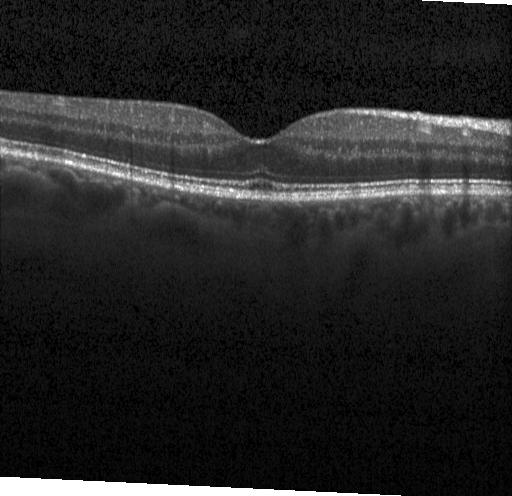

Heidelberg Spectralis OCT system · spectral-domain OCT · horizontal scan through the fovea · OCT line scan — Assessment: no CNV, DME, or drusen.